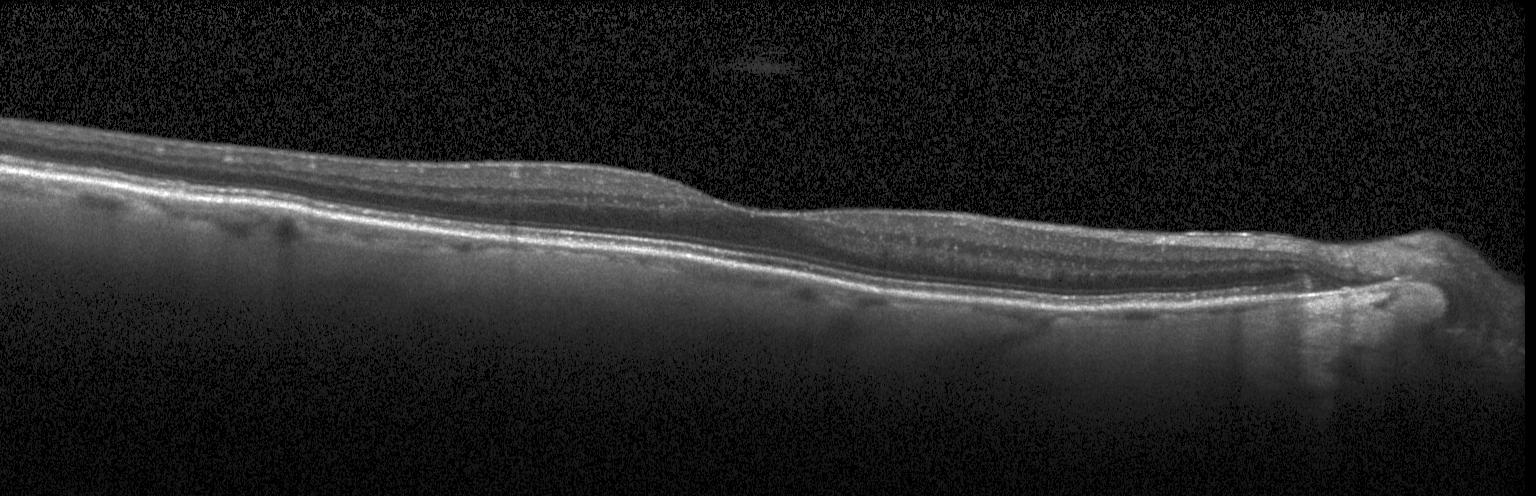

OCT B-scan, spectral-domain optical coherence tomography — Finding: neither CNV, DME, nor drusen.